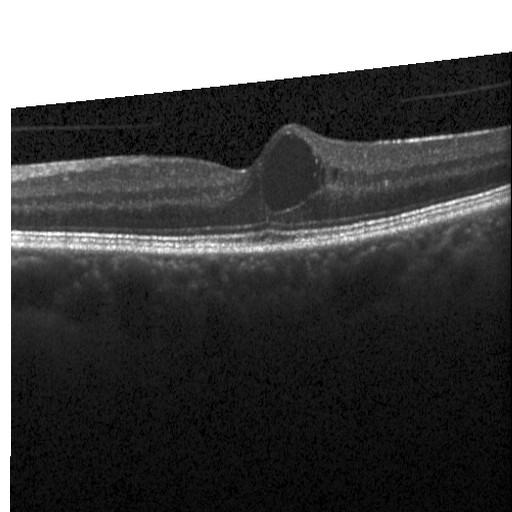
SD-OCT. Acquired on a Heidelberg Spectralis. Optical coherence tomography scan
Diagnosis: diabetic macular edema (DME).